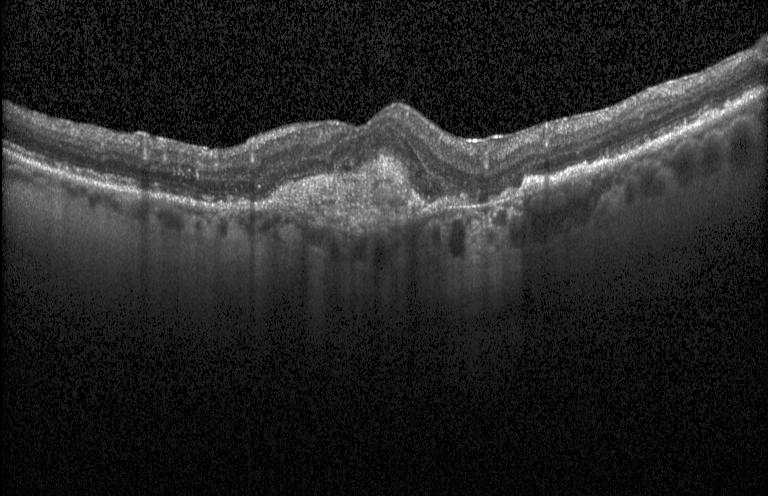 Instrument: Heidelberg Spectralis; retinal OCT cross-section — Finding: a choroidal neovascular membrane.